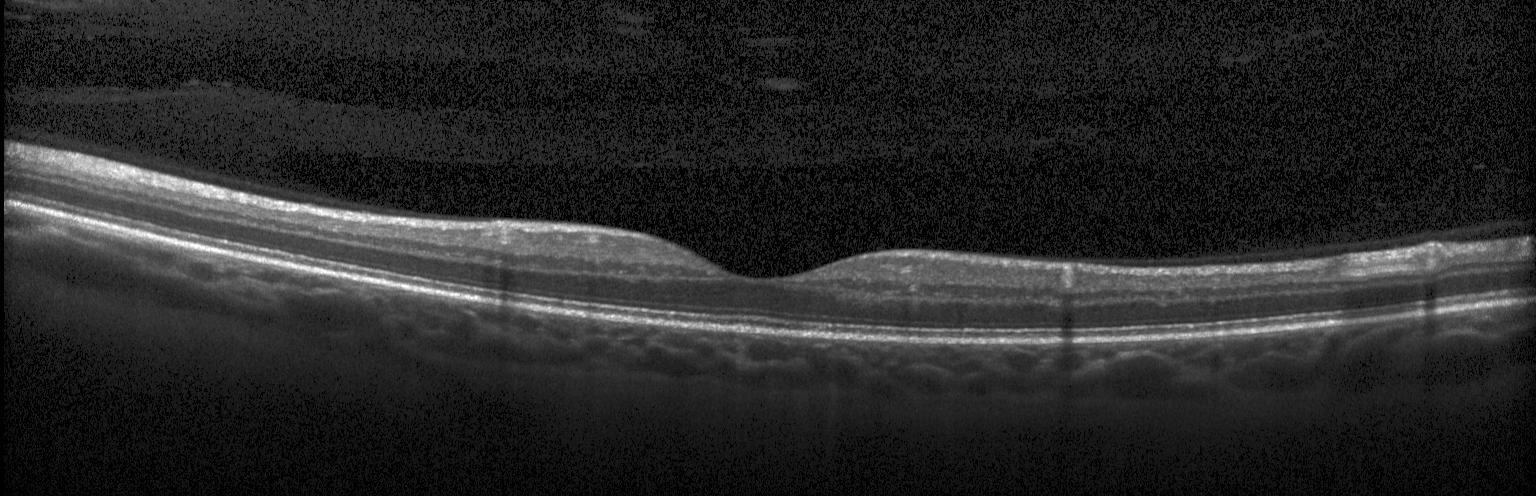 Optical coherence tomography scan. Heidelberg Spectralis. Fovea-centered. Spectral-domain OCT. Impression: no choroidal neovascularization, diabetic macular edema, or drusen.